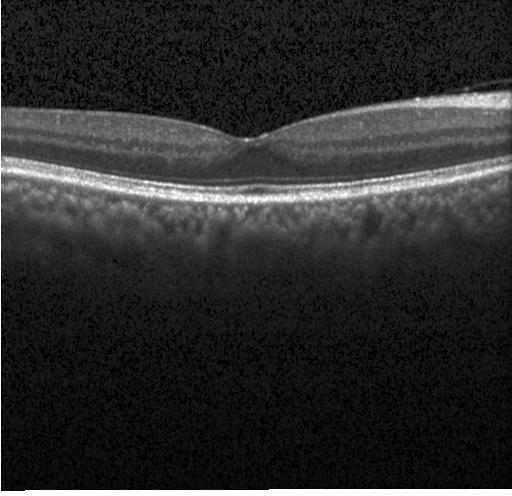
Centered on the fovea, Heidelberg Spectralis OCT system, OCT B-scan, spectral-domain optical coherence tomography
Assessment: no CNV, DME, or drusen.